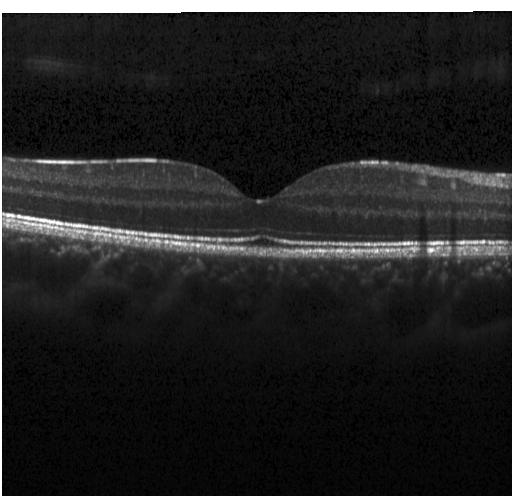

Assessment: no evidence of CNV, DME, or drusen.